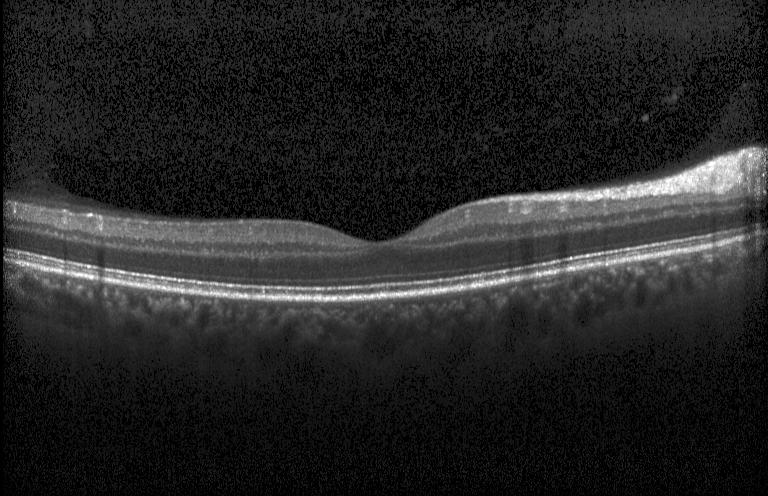

Retinal OCT cross-section.
Impression: no CNV, DME, or drusen.